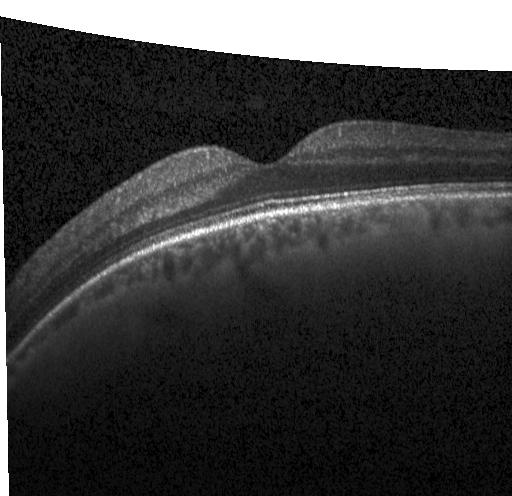
Finding: no choroidal neovascularization, diabetic macular edema, or drusen.